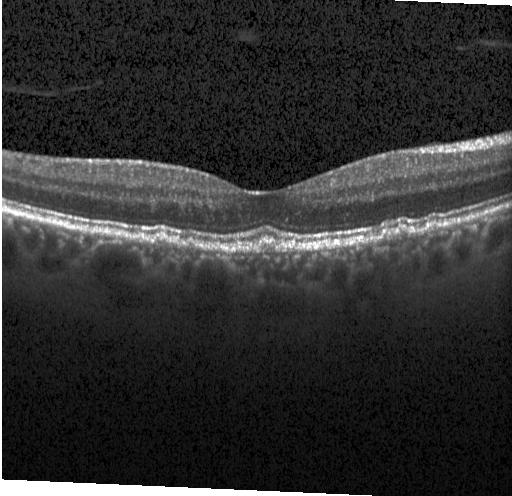 Macular OCT demonstrating sub-RPE drusenoid deposits.